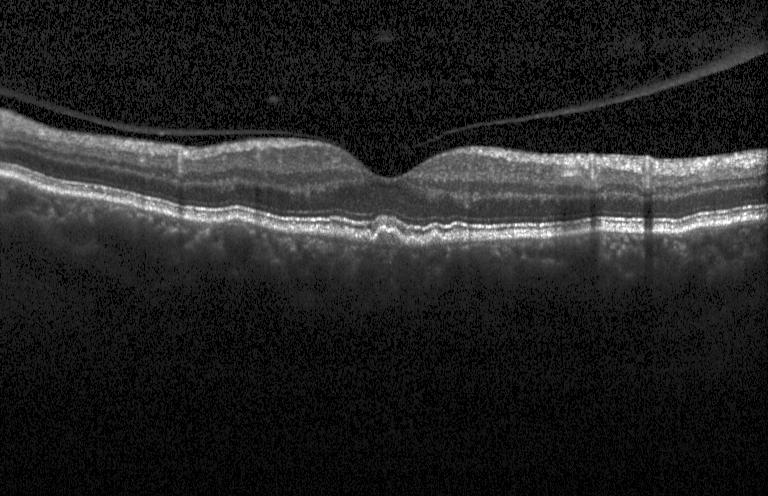
Spectral-domain optical coherence tomography. Heidelberg Spectralis. Retinal OCT cross-section.
Diagnosis: sub-RPE drusenoid deposits.